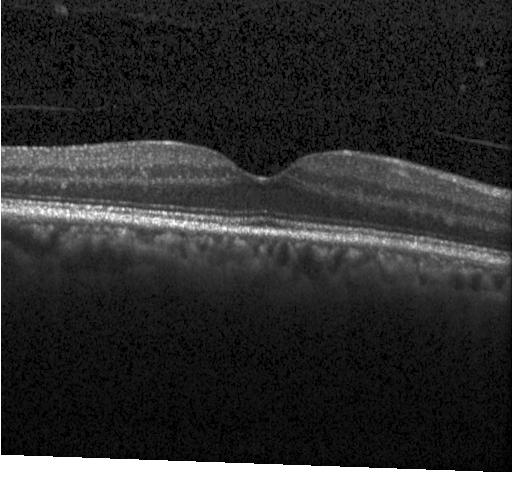

Optical coherence tomography B-scan. SD-OCT. Horizontal scan through the fovea
Assessment: no choroidal neovascularization, diabetic macular edema, or drusen.